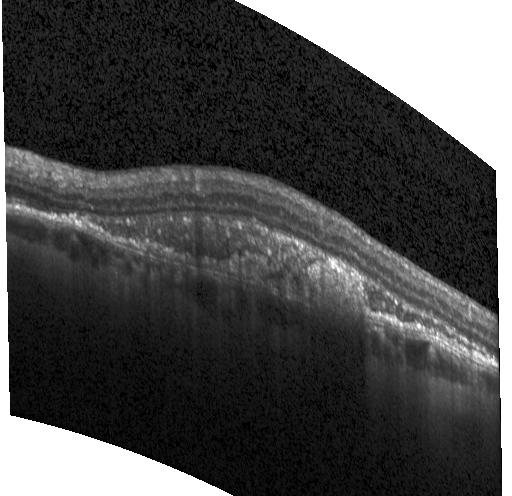 Retinal OCT cross-section.
OCT finding: choroidal neovascularization (CNV).